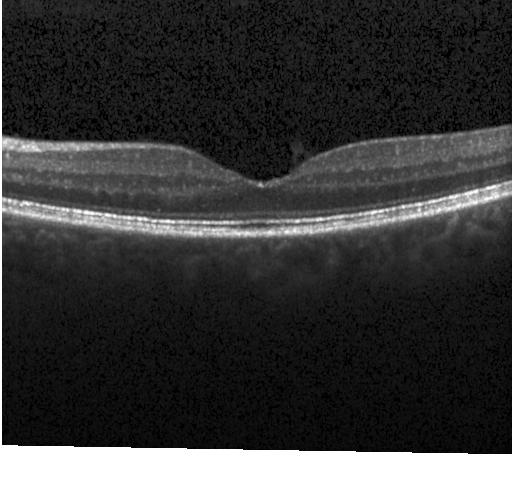

Dx: neither choroidal neovascularization, diabetic macular edema, nor drusen.